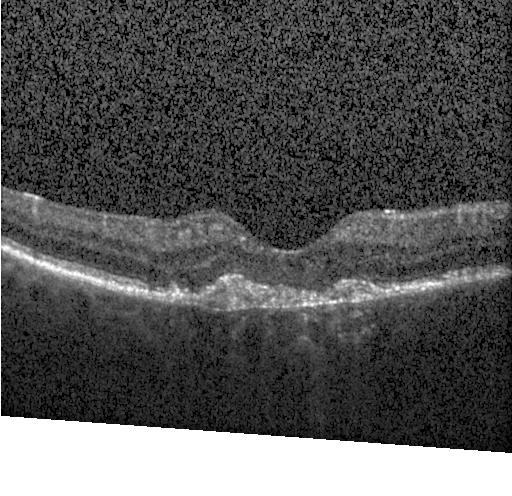
A choroidal neovascular membrane.